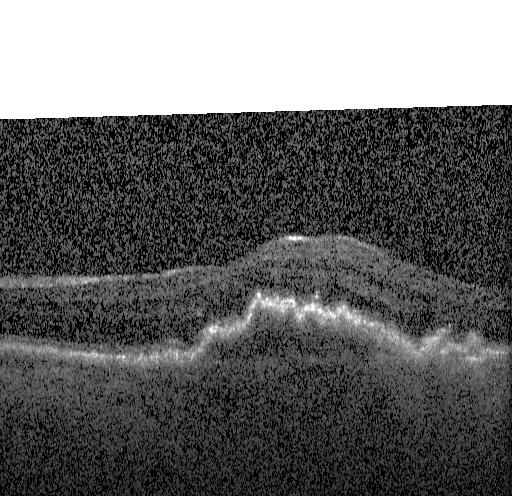
A choroidal neovascular membrane.